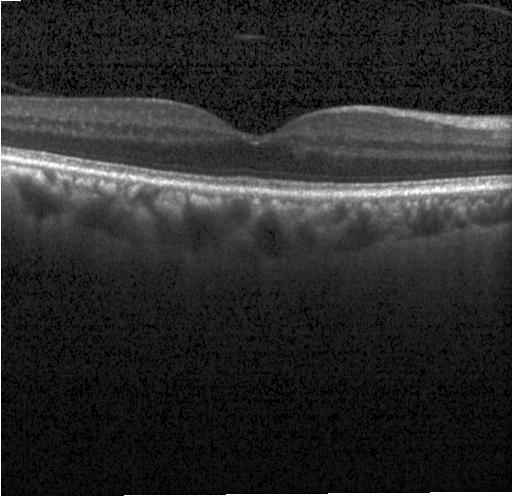
OCT B-scan; spectral-domain optical coherence tomography; Heidelberg Spectralis; centered on the fovea
Diagnosis: no evidence of choroidal neovascularization, diabetic macular edema, or drusen.